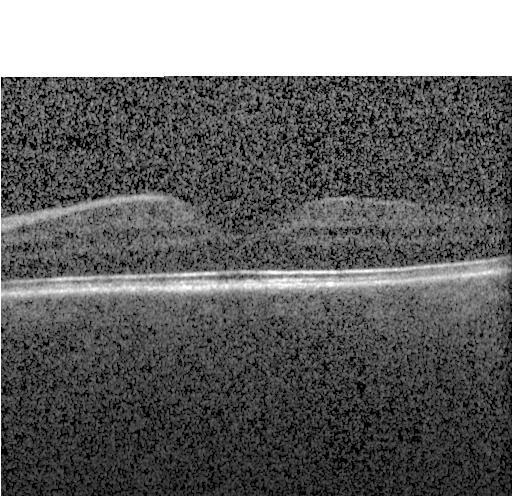
Optical coherence tomography scan.
Dx: no evidence of choroidal neovascularization, diabetic macular edema, or drusen.